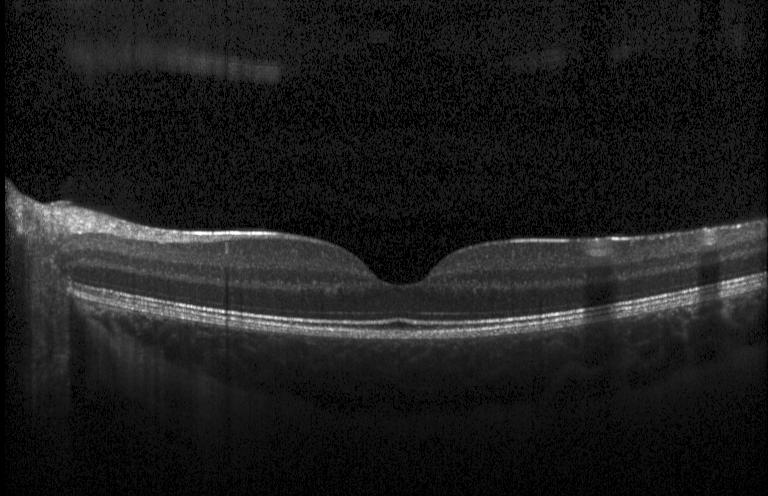
Through the macula, OCT B-scan
Finding: no choroidal neovascularization, diabetic macular edema, or drusen.